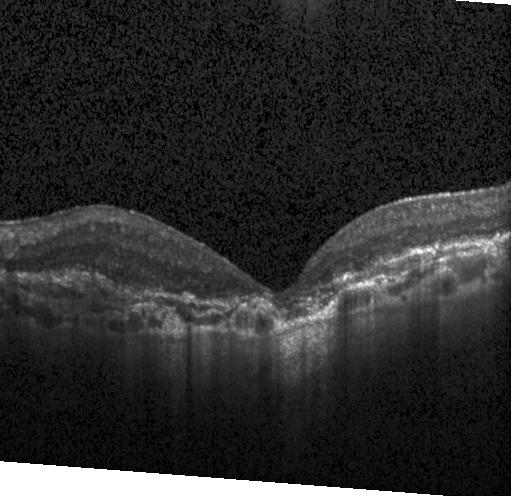

This B-scan demonstrates choroidal neovascularization.